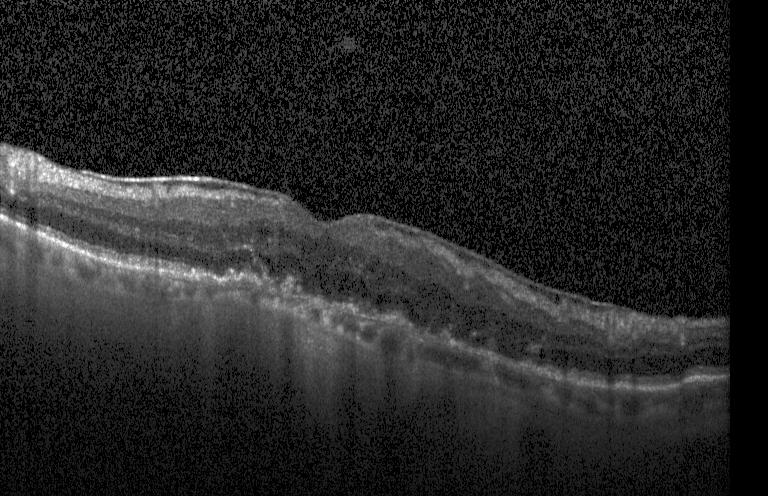 Through the macula; Heidelberg Spectralis OCT system; SD-OCT; retinal OCT B-scan
Finding: CNV.